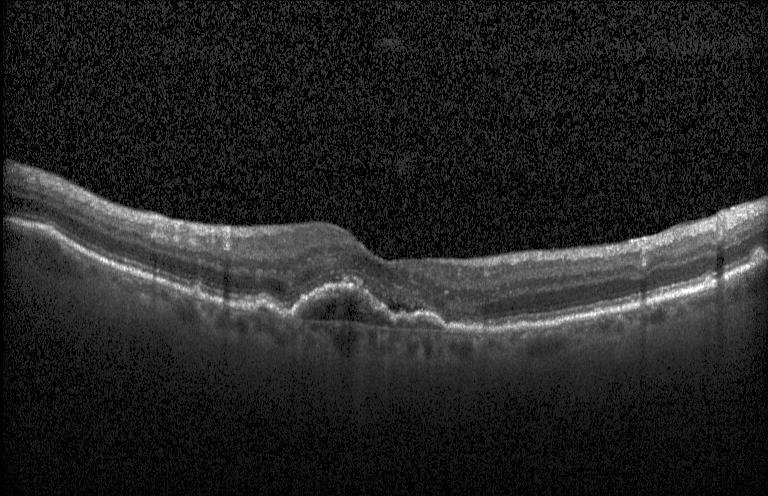

Retinal OCT B-scan
This B-scan demonstrates CNV.